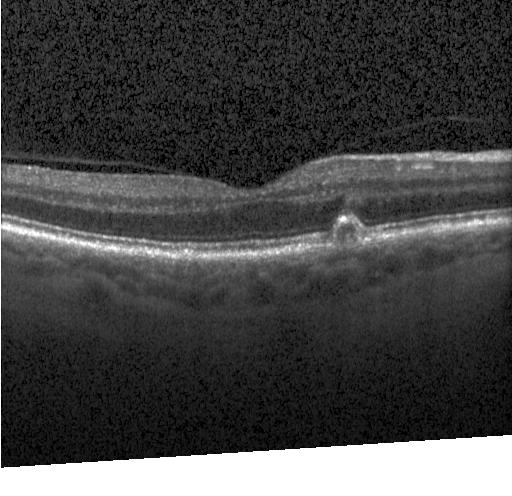 OCT B-scan showing drusen.